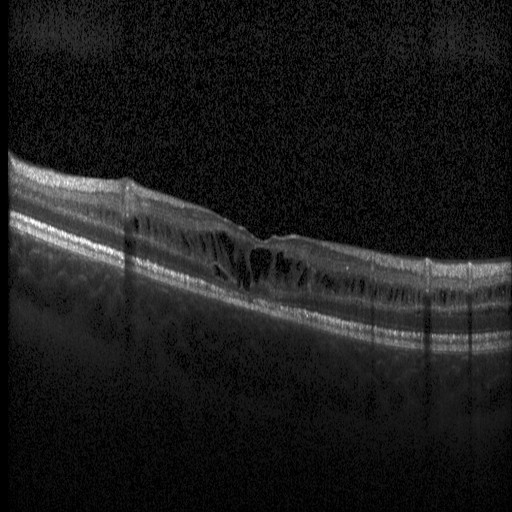
Retinal OCT B-scan. Diagnosis: diabetic macular edema.